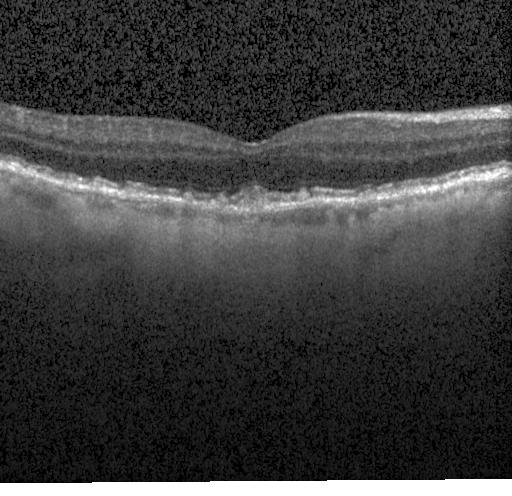
Retinal OCT B-scan; macular scan — Diagnosis: sub-RPE drusenoid deposits.